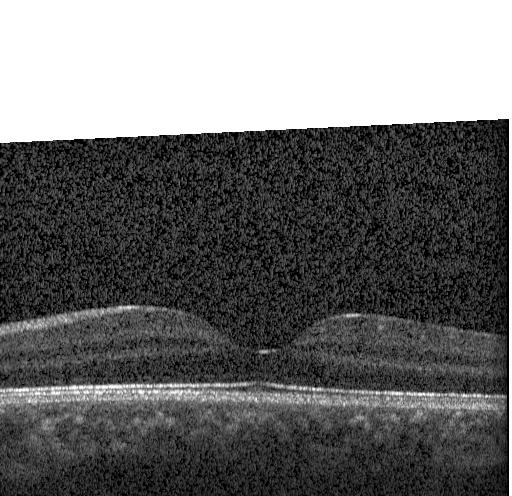 Fovea-centered, optical coherence tomography B-scan. The scan shows no CNV, no DME, and no drusen.